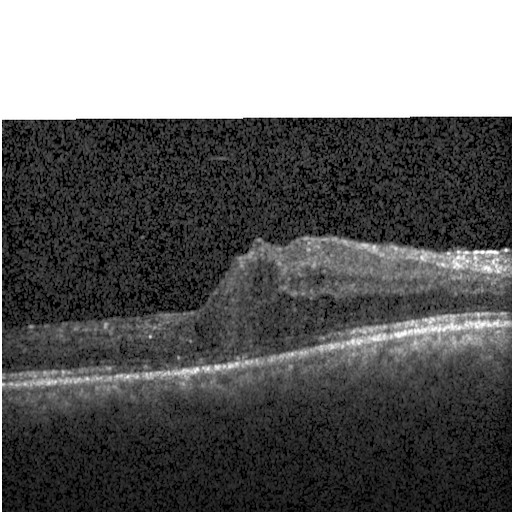 Macular scan. Retinal OCT cross-section. Impression: diabetic macular edema.